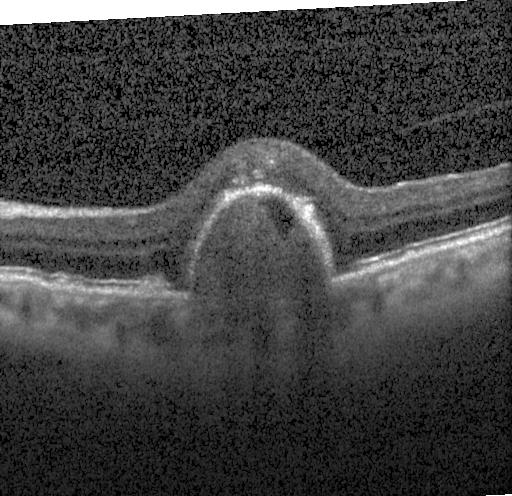
Impression: a choroidal neovascular membrane.